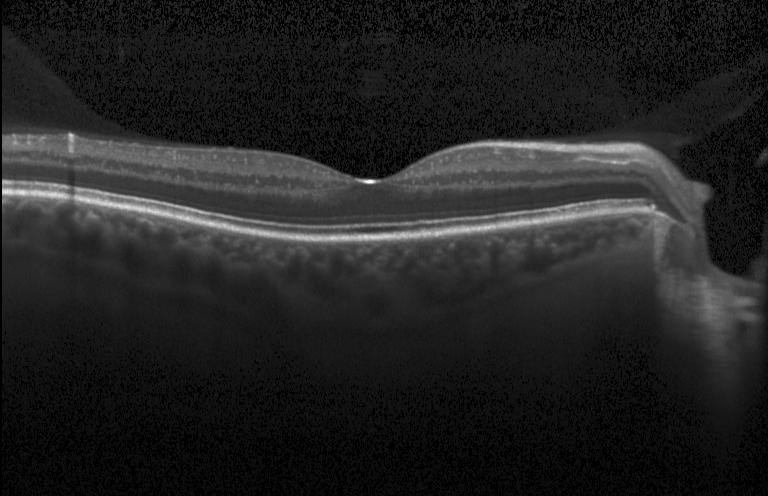 Retinal OCT B-scan. Heidelberg Spectralis
Assessment: no evidence of CNV, DME, or drusen.